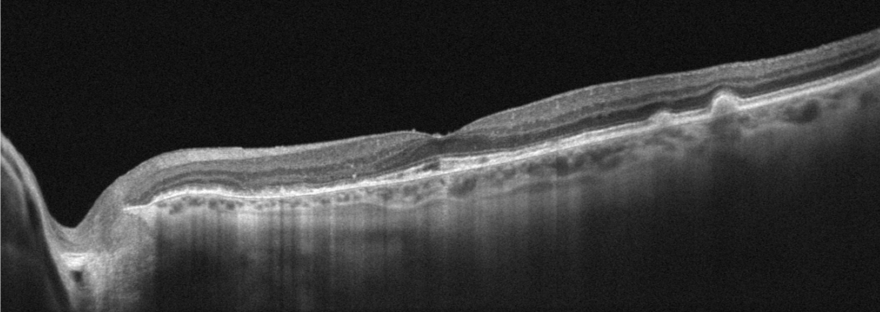

Retinal OCT cross-section.
OCT finding: age-related macular degeneration (AMD).